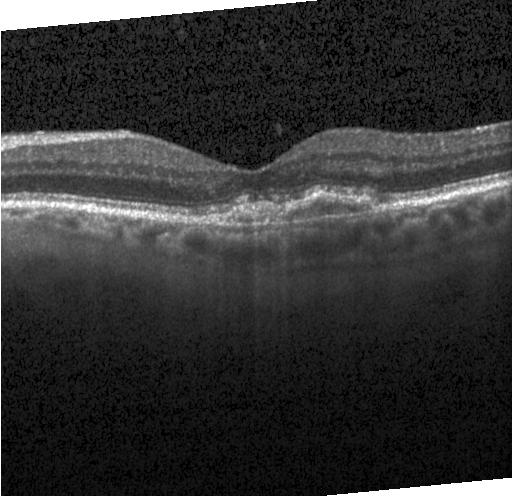
Macular OCT: choroidal neovascularization.